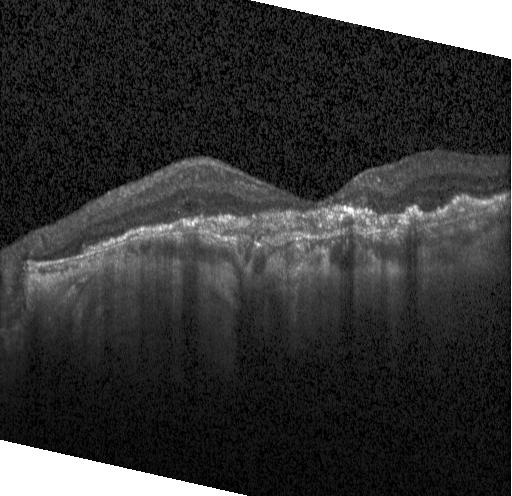

Choroidal neovascularization.